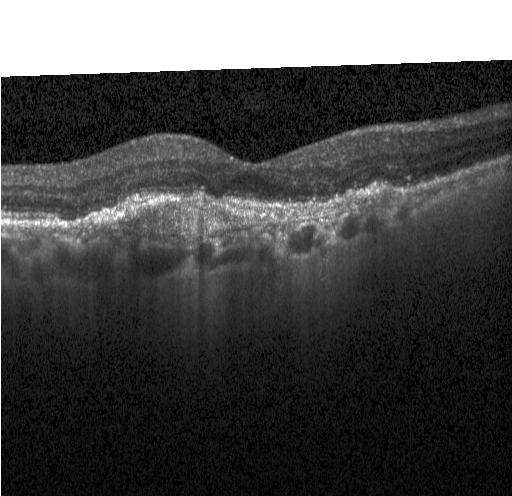 The scan shows choroidal neovascularization.